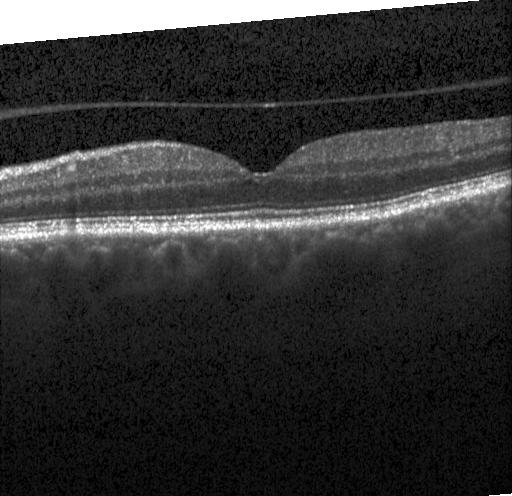
Retinal OCT B-scan; Heidelberg Spectralis OCT system.
The scan shows no choroidal neovascularization, diabetic macular edema, or drusen.